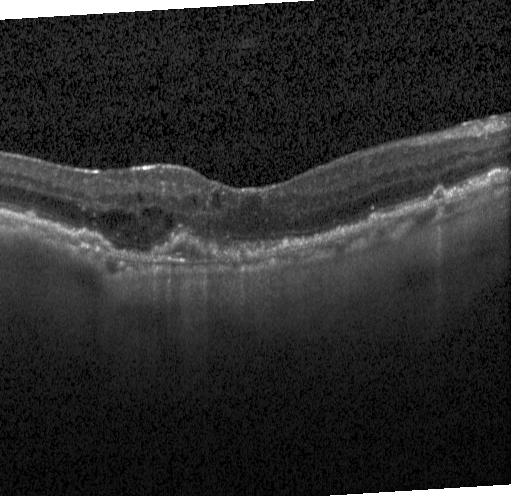 OCT line scan — Finding: CNV.